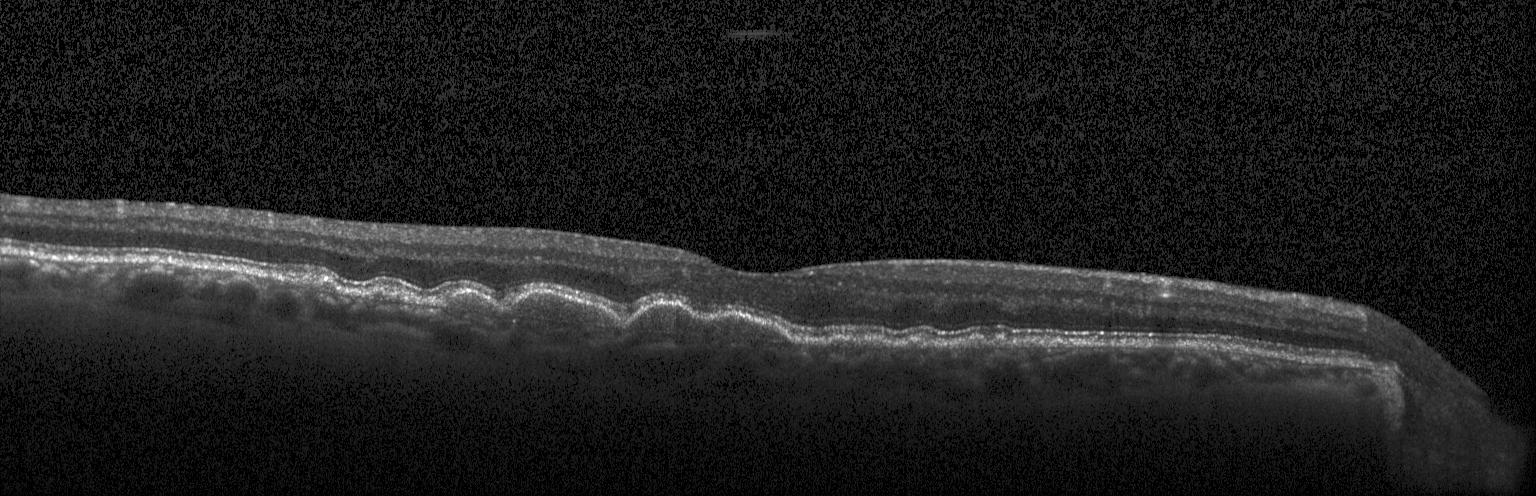

Dx: multiple drusen.